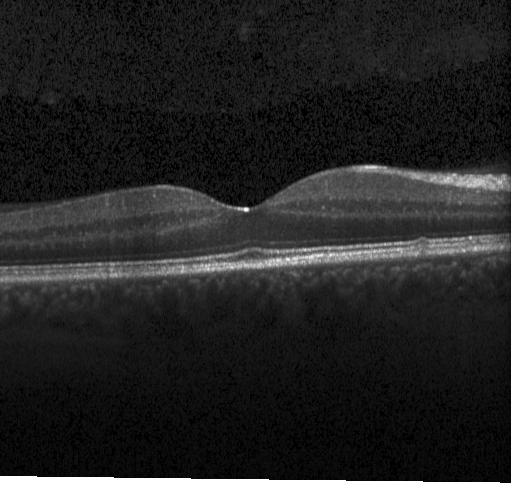
No evidence of CNV, DME, or drusen.